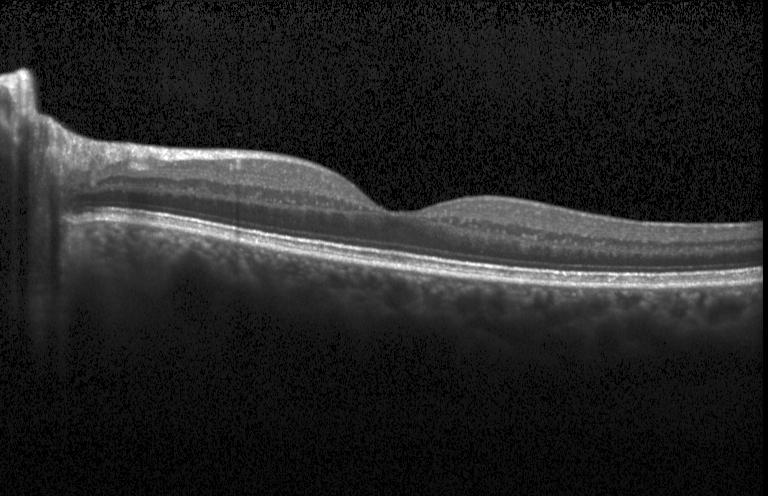 Acquired on a Heidelberg Spectralis. OCT line scan — Macular OCT: no choroidal neovascularization, diabetic macular edema, or drusen.